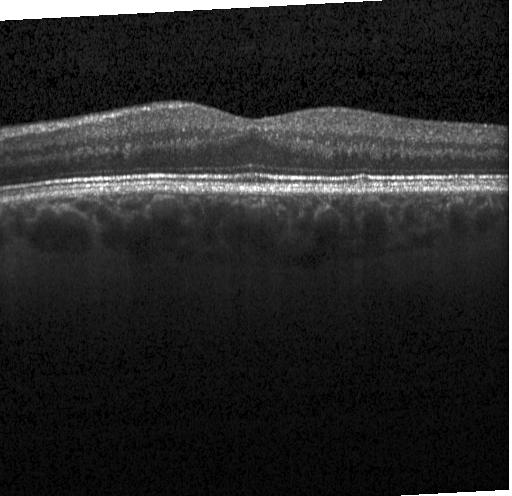 Diagnosis: no choroidal neovascularization, no diabetic macular edema, and no drusen.